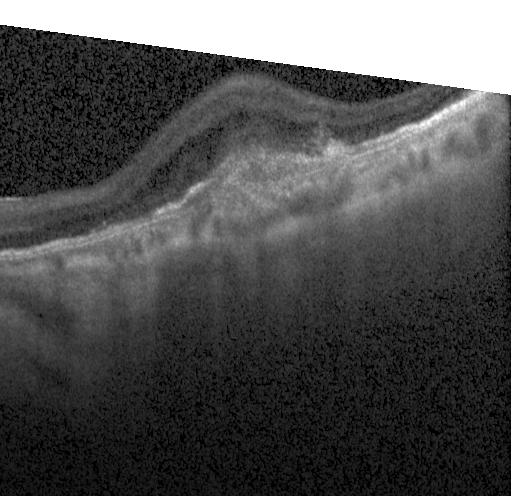
Finding: a choroidal neovascular membrane.